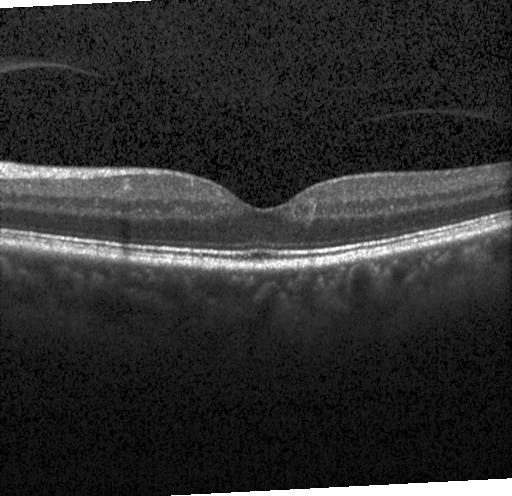 Spectral-domain OCT · macular scan · OCT B-scan.
Finding: no evidence of choroidal neovascularization, diabetic macular edema, or drusen.